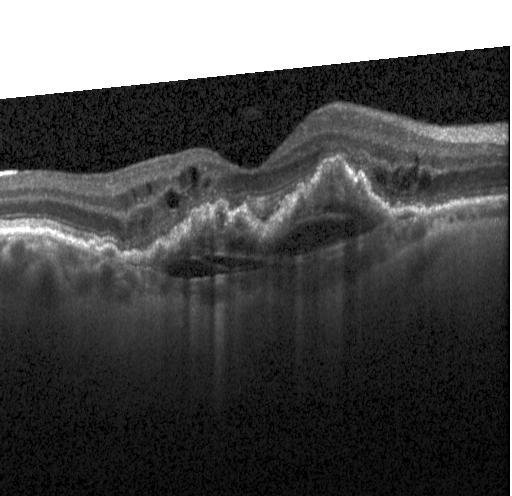
Impression: CNV.